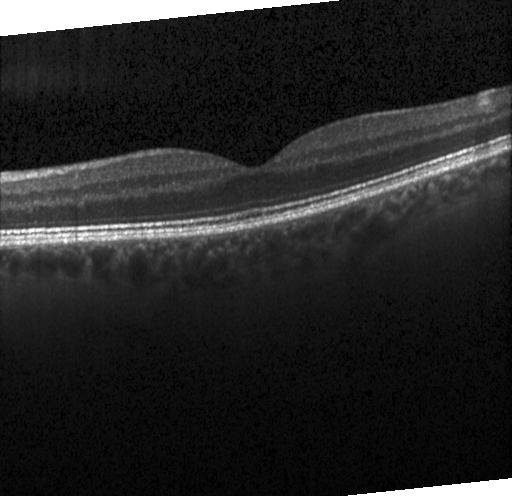

Finding: neither choroidal neovascularization, diabetic macular edema, nor drusen.